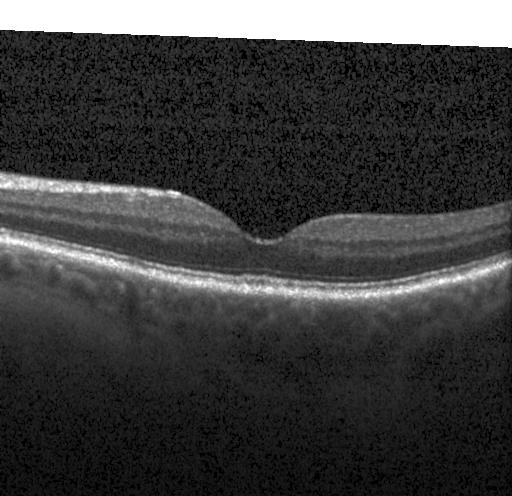
OCT line scan; Heidelberg Spectralis; SD-OCT — No evidence of choroidal neovascularization, diabetic macular edema, or drusen.